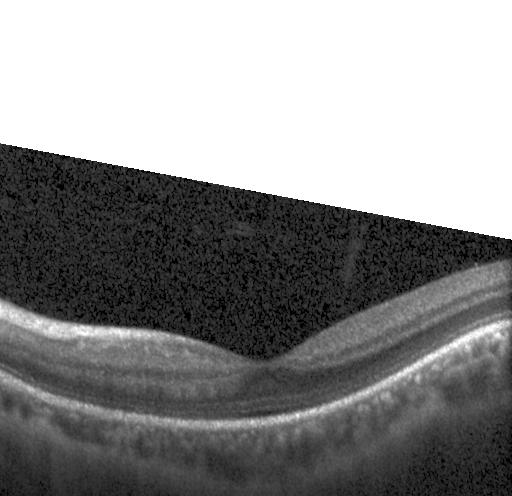
Spectral-domain OCT B-scan: no evidence of CNV, DME, or drusen.